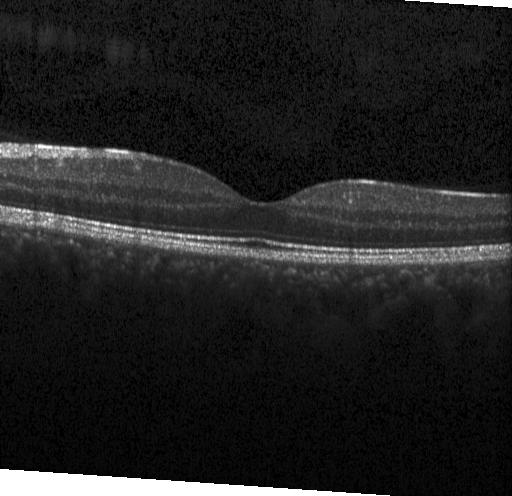
Retinal OCT cross-section showing no choroidal neovascularization, diabetic macular edema, or drusen.